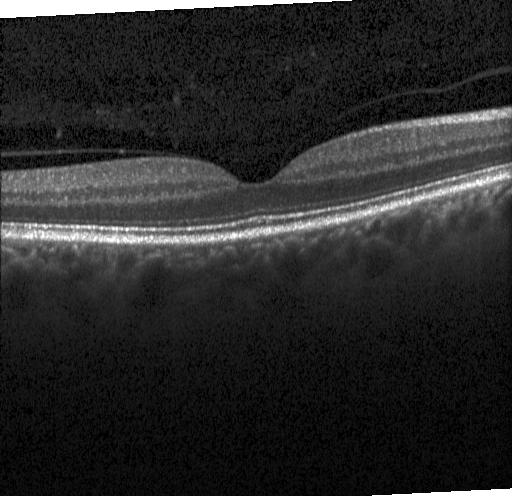

Optical coherence tomography B-scan; Heidelberg Spectralis OCT system.
Dx: neither choroidal neovascularization, diabetic macular edema, nor drusen.